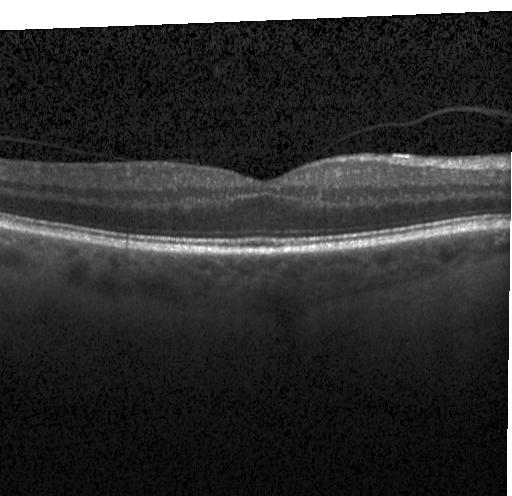 OCT B-scan; SD-OCT.
Finding: no choroidal neovascularization, diabetic macular edema, or drusen.